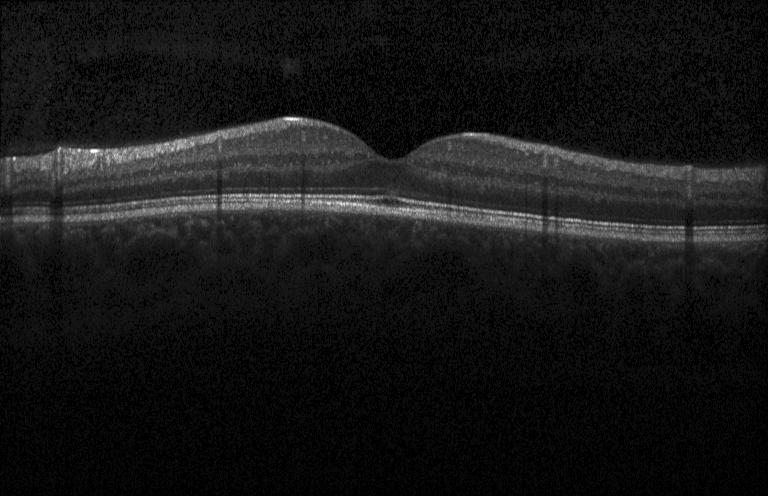

Retinal OCT B-scan.
Impression: neither CNV, DME, nor drusen.